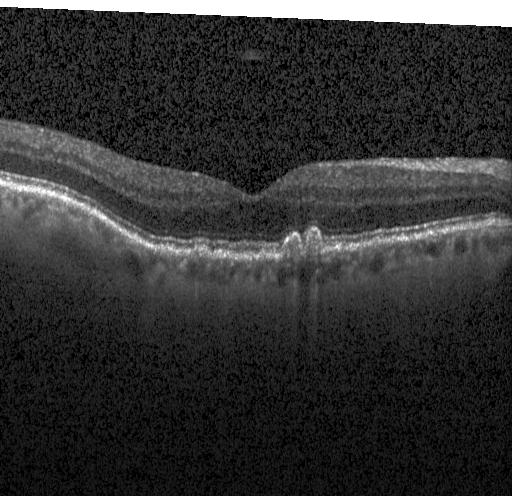
Diagnosis: drusen.